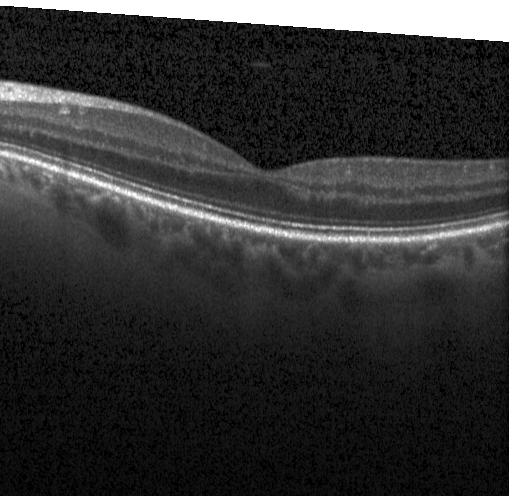

Impression: no choroidal neovascularization, diabetic macular edema, or drusen.